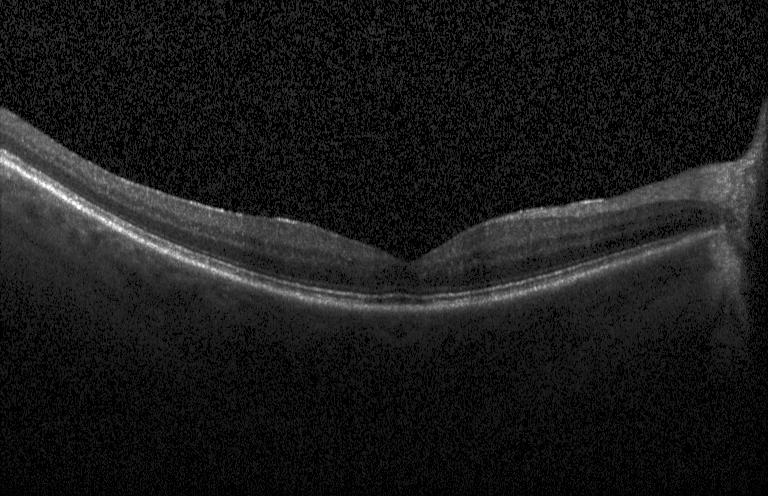
OCT finding: no choroidal neovascularization, no diabetic macular edema, and no drusen.